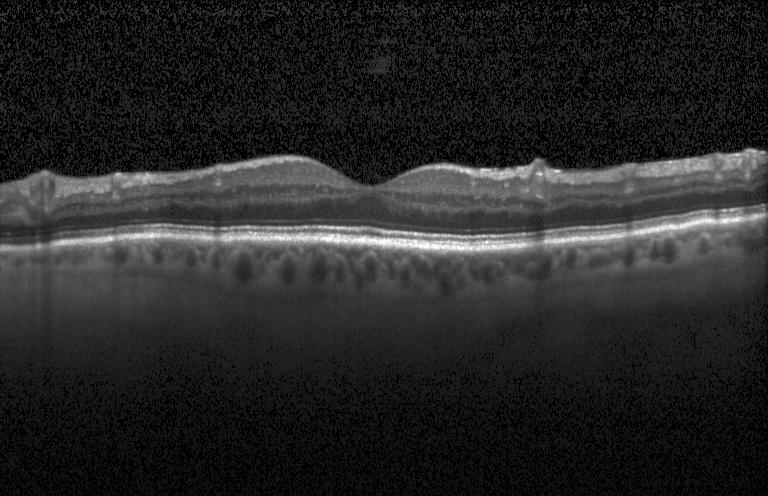
OCT line scan
Finding: no choroidal neovascularization, diabetic macular edema, or drusen.